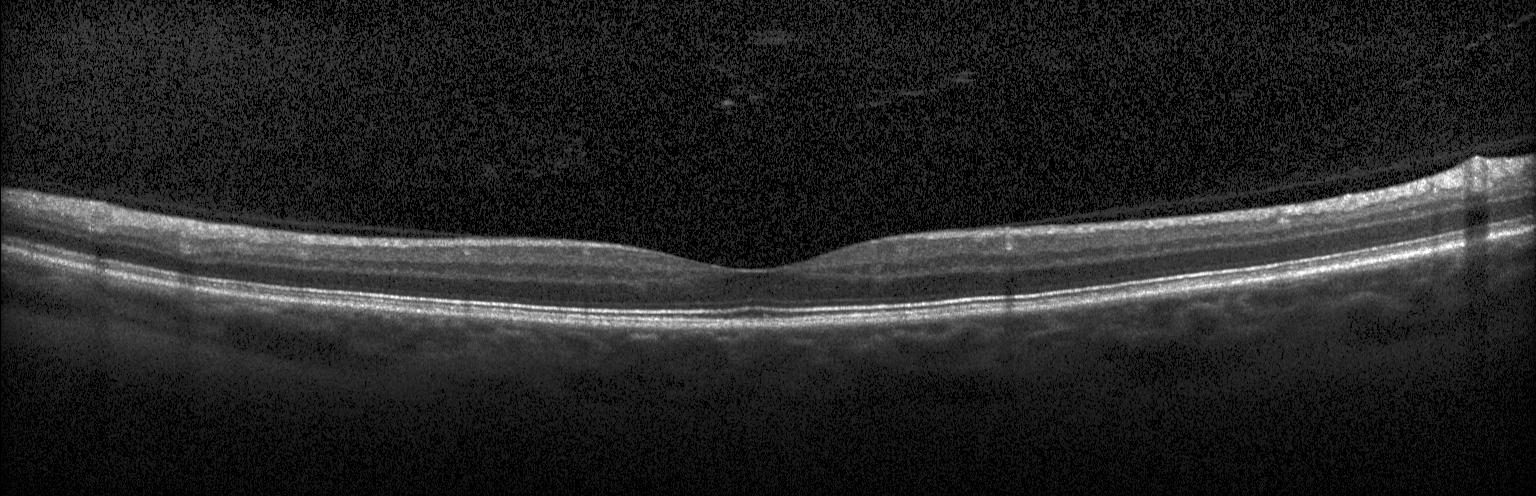

Horizontal scan through the fovea; instrument: Heidelberg Spectralis; OCT B-scan; spectral-domain OCT.
OCT finding: no choroidal neovascularization, diabetic macular edema, or drusen.